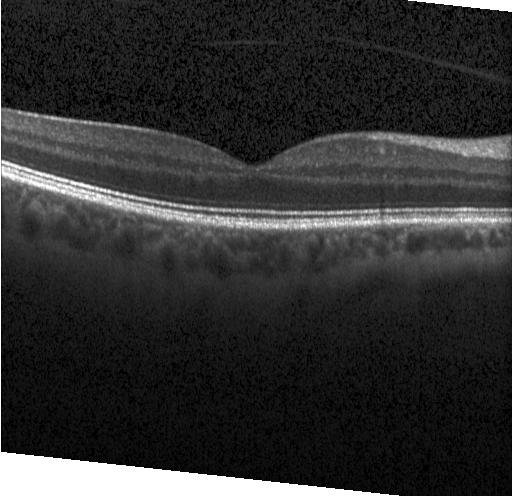 OCT B-scan; instrument: Heidelberg Spectralis; spectral-domain optical coherence tomography; centered on the fovea — Macular OCT: neither choroidal neovascularization, diabetic macular edema, nor drusen.